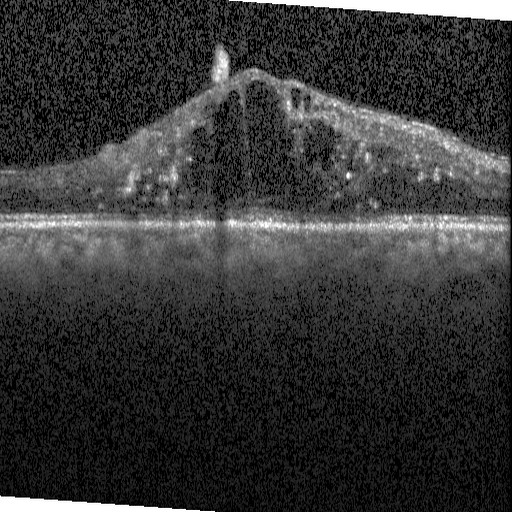
OCT finding: diabetic macular edema (DME).